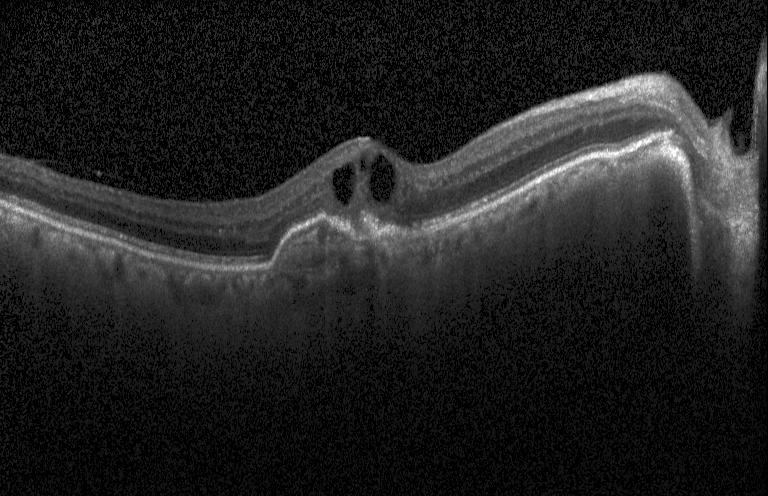

Spectral-domain OCT B-scan: a choroidal neovascular membrane.